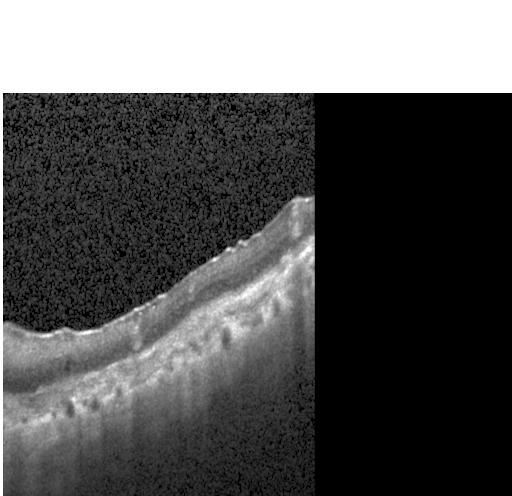

Instrument: Heidelberg Spectralis; OCT line scan; macular scan; SD-OCT. CNV.